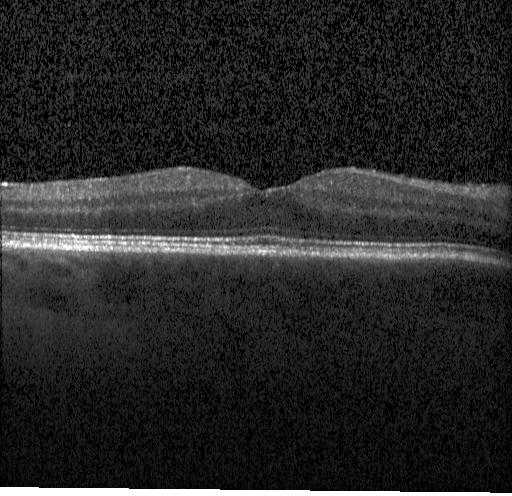

This B-scan demonstrates no CNV, DME, or drusen.